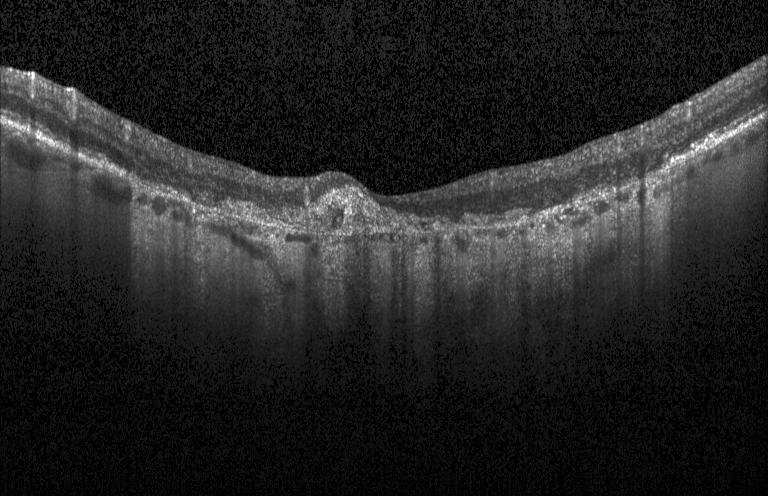

Spectral-domain OCT B-scan: CNV.